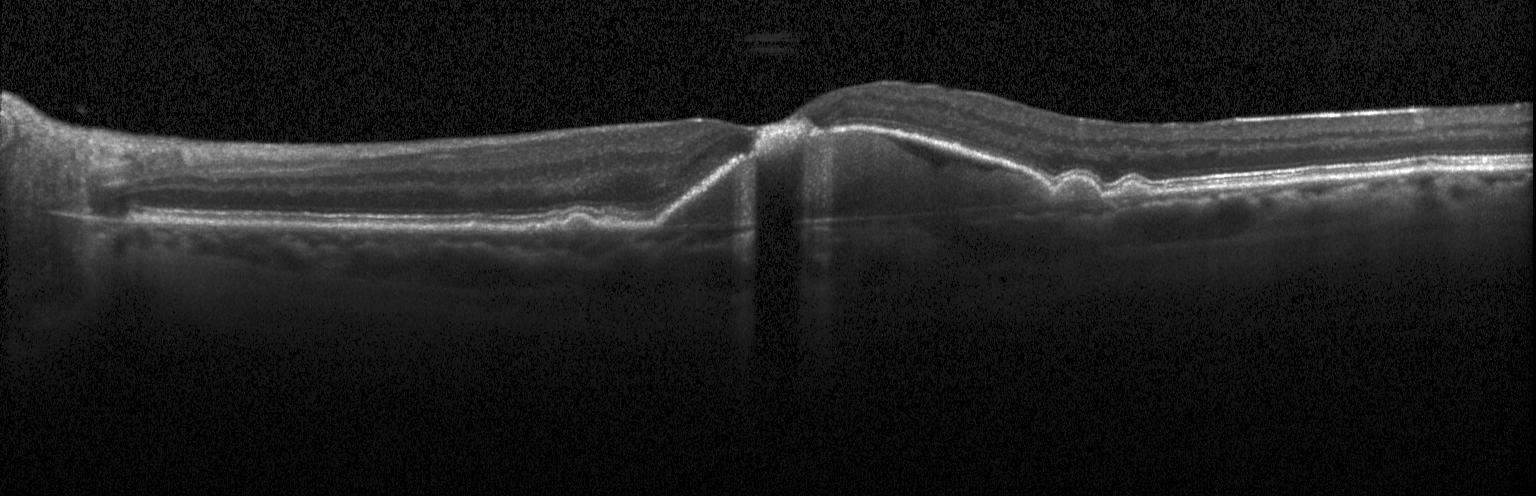
Horizontal scan through the fovea · optical coherence tomography scan — Finding: a choroidal neovascular membrane.